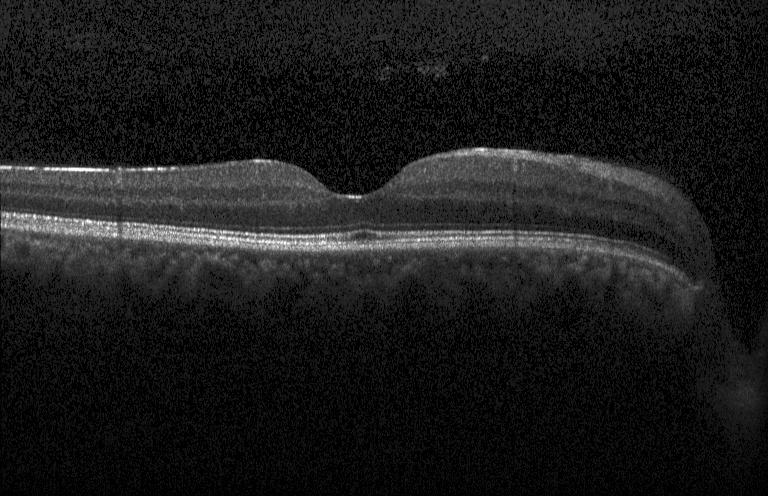
Spectral-domain OCT B-scan: no evidence of choroidal neovascularization, diabetic macular edema, or drusen.